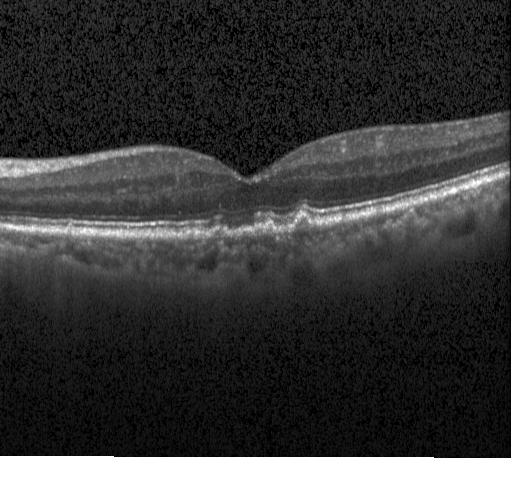 Retinal OCT cross-section. Fovea-centered. SD-OCT — Diagnosis: multiple drusen.